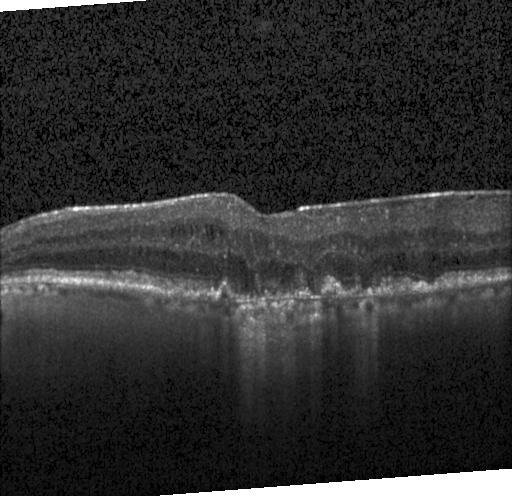
Finding: choroidal neovascularization.